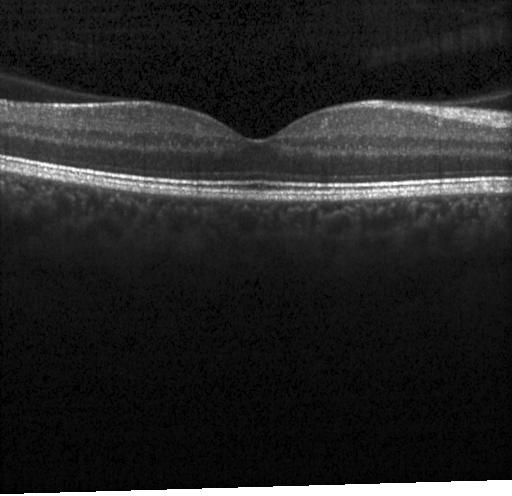 Diagnosis: no choroidal neovascularization, diabetic macular edema, or drusen.